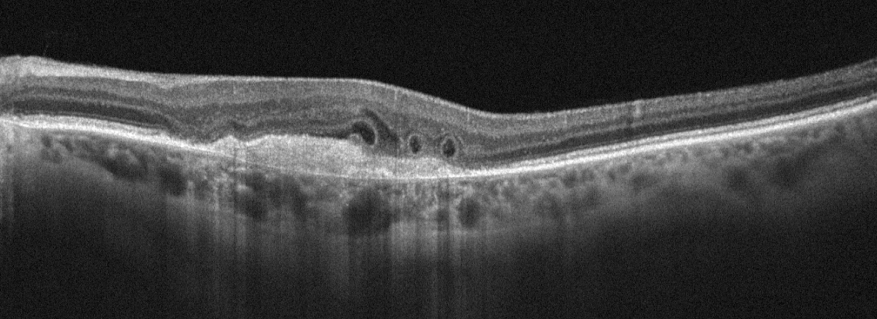 Optical coherence tomography B-scan.
The scan shows age-related macular degeneration (AMD).